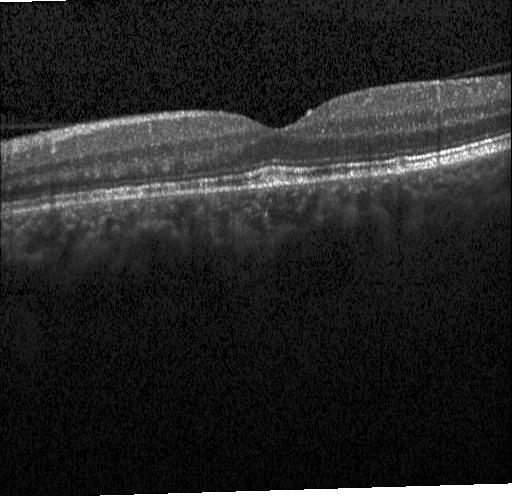
Optical coherence tomography B-scan.
The scan shows no choroidal neovascularization, diabetic macular edema, or drusen.